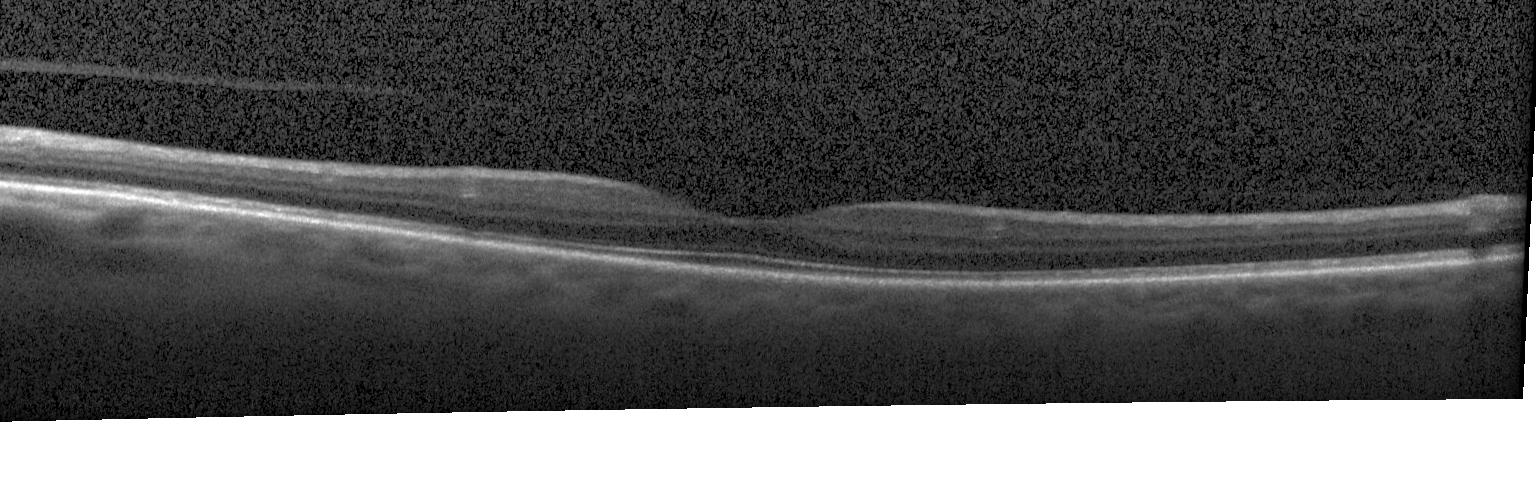
Spectral-domain optical coherence tomography. Optical coherence tomography B-scan. Acquired on a Heidelberg Spectralis.
Diagnosis: no choroidal neovascularization, diabetic macular edema, or drusen.